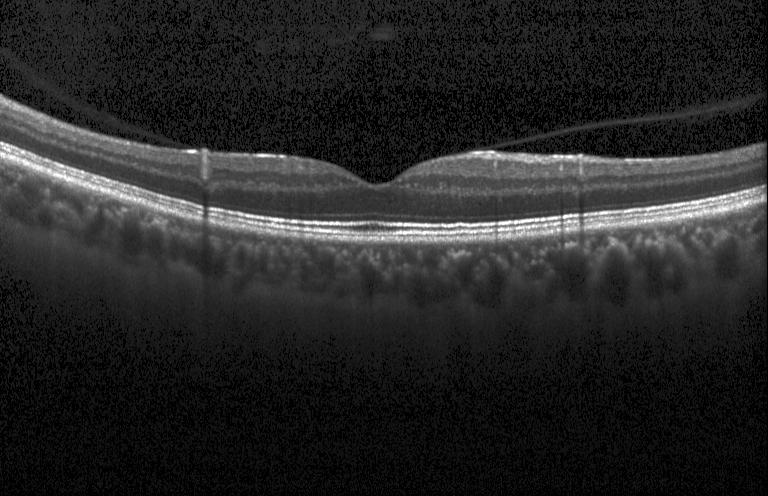
Retinal OCT B-scan · centered on the fovea.
Assessment: no CNV, no DME, and no drusen.